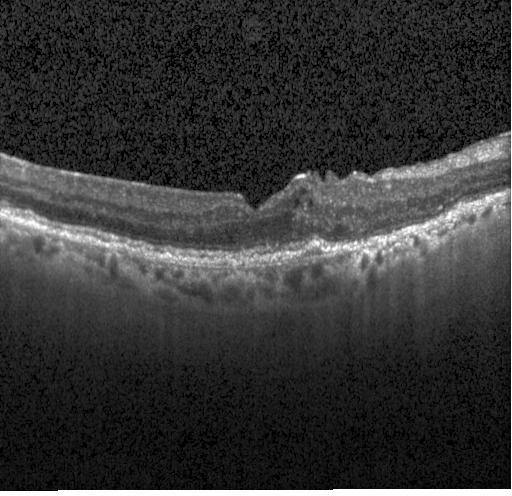 Heidelberg Spectralis; SD-OCT; through the macula; retinal OCT cross-section — Macular OCT: a choroidal neovascular membrane.